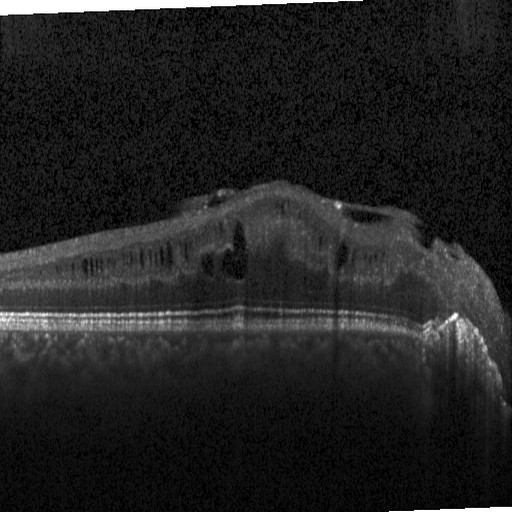

Through the macula; Heidelberg Spectralis OCT system; optical coherence tomography scan. Impression: DME.